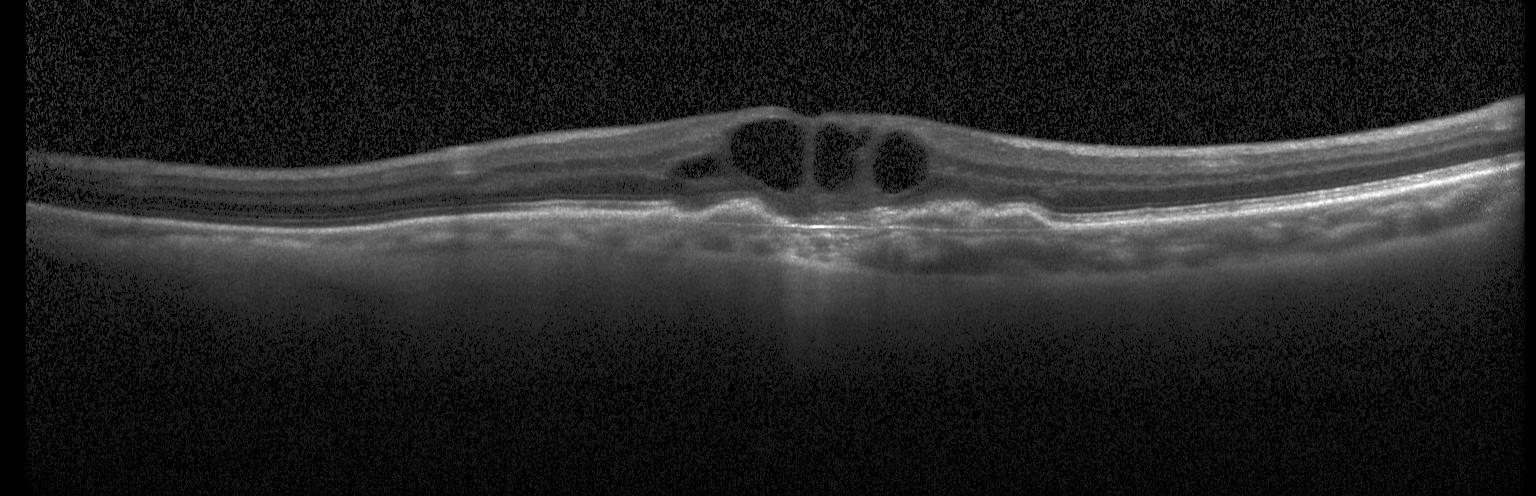

The scan shows a choroidal neovascular membrane.